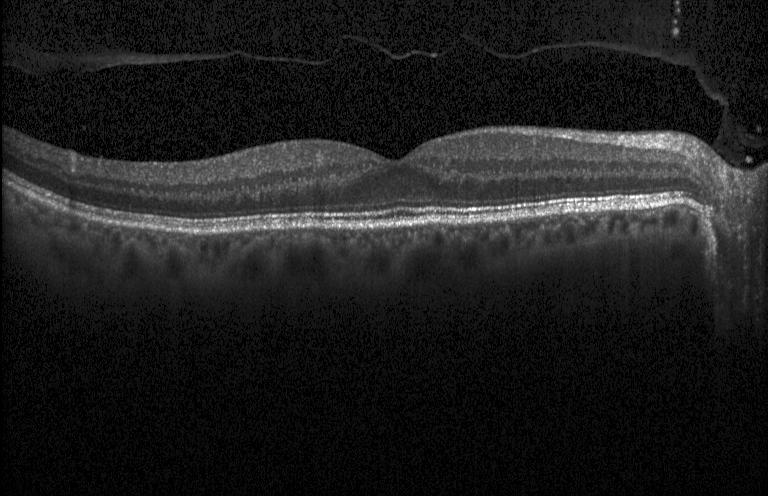 OCT line scan — Assessment: no CNV, no DME, and no drusen.